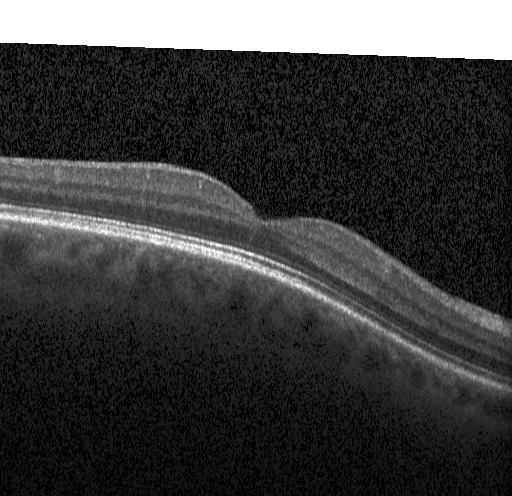
Diagnosis: no choroidal neovascularization, diabetic macular edema, or drusen.